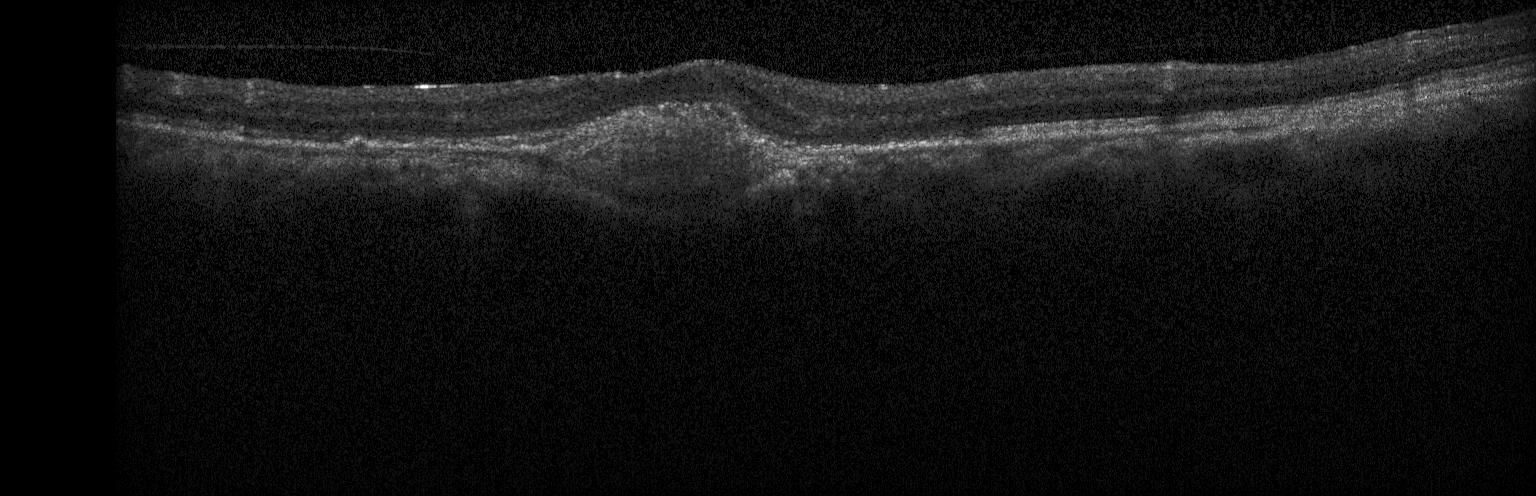 Fovea-centered, retinal OCT cross-section, instrument: Heidelberg Spectralis — Macular OCT: a choroidal neovascular membrane.